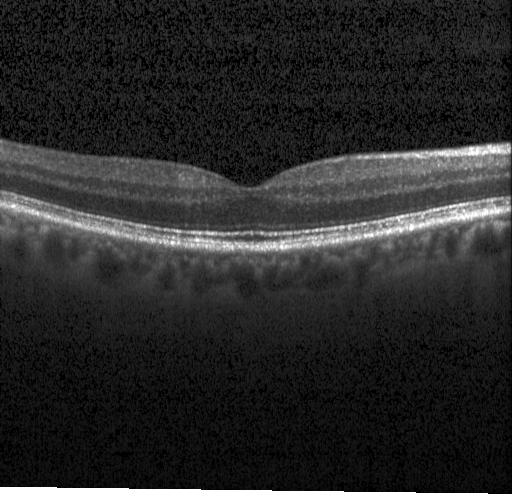 Retinal OCT B-scan; Heidelberg Spectralis OCT system; through the macula; spectral-domain optical coherence tomography
Impression: no choroidal neovascularization, no diabetic macular edema, and no drusen.